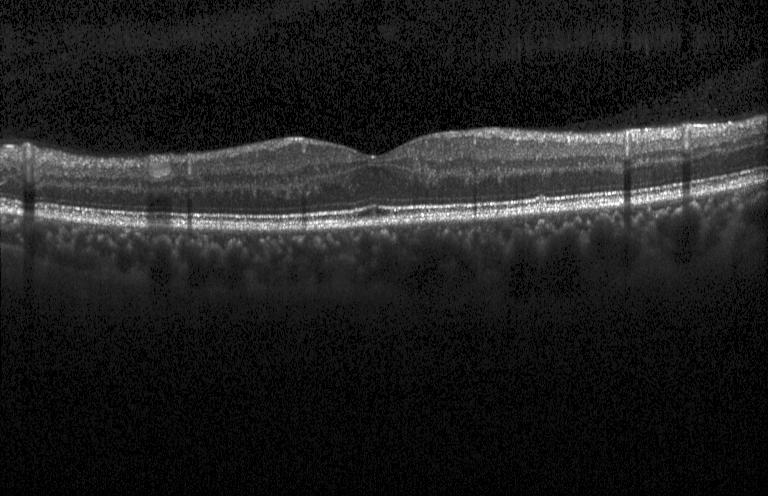
Through the macula. Heidelberg Spectralis OCT system. OCT line scan. Spectral-domain optical coherence tomography
Diagnosis: no evidence of choroidal neovascularization, diabetic macular edema, or drusen.